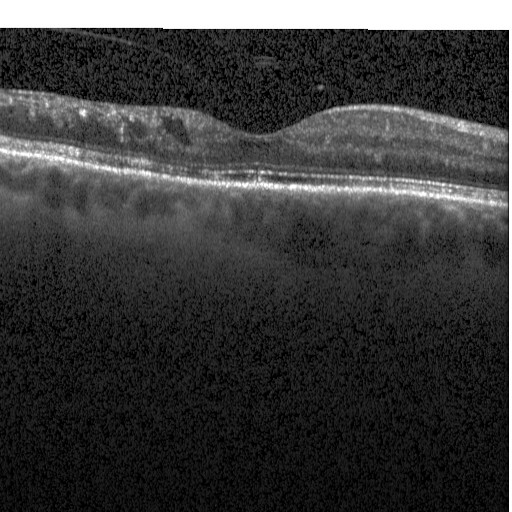

Macular OCT: diabetic macular edema.